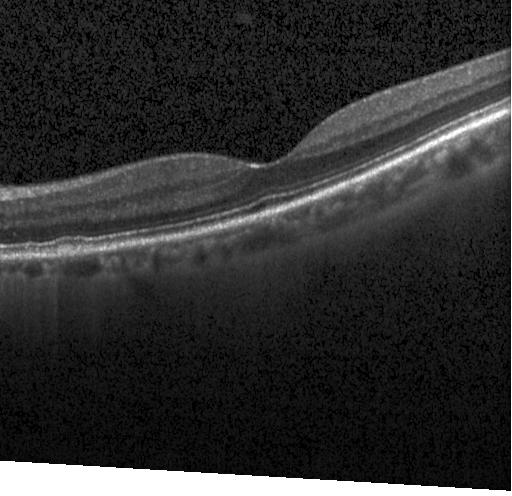 OCT finding: no choroidal neovascularization, diabetic macular edema, or drusen.